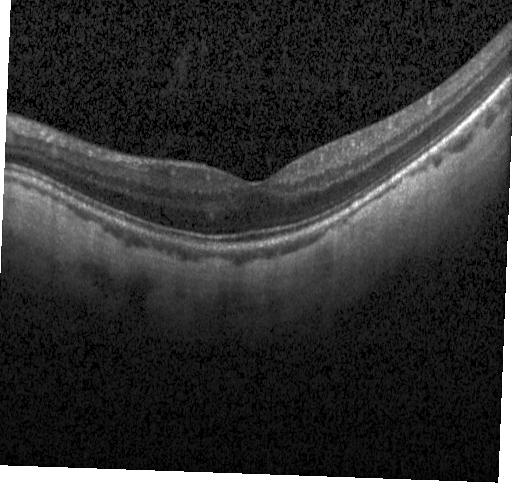
Heidelberg Spectralis OCT system · SD-OCT · retinal OCT B-scan · centered on the fovea
Finding: no evidence of choroidal neovascularization, diabetic macular edema, or drusen.